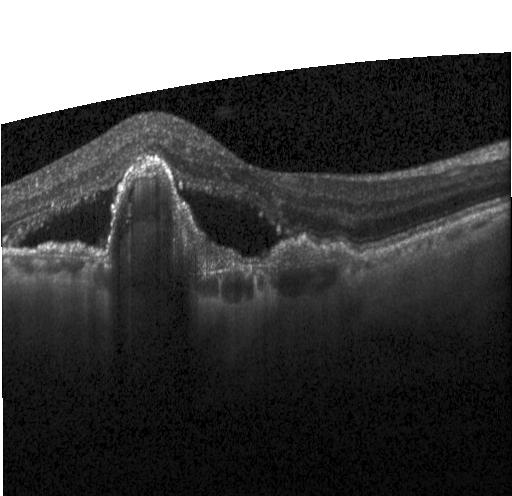
Retinal OCT cross-section — Dx: choroidal neovascularization (CNV).